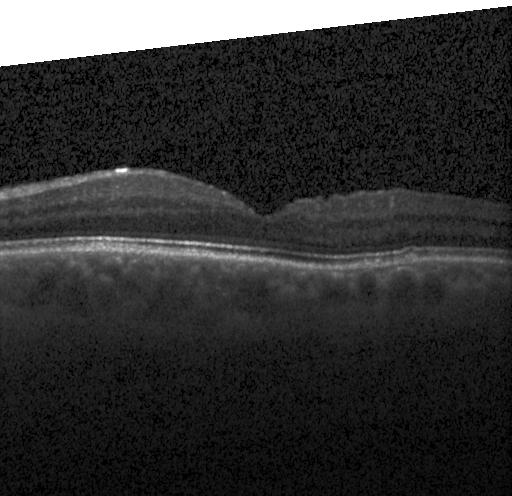

Retinal OCT cross-section, spectral-domain OCT
Diagnosis: no evidence of CNV, DME, or drusen.